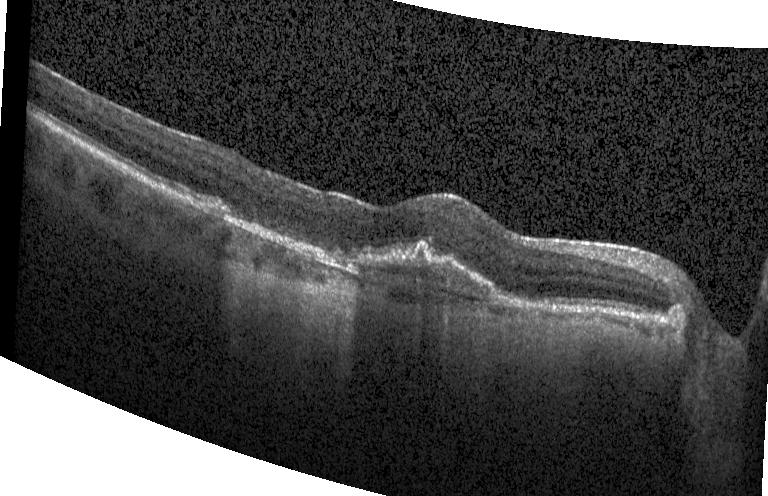
Macular OCT: CNV.